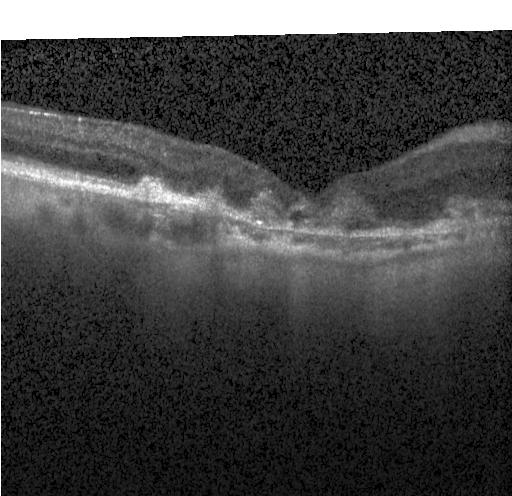 Retinal OCT cross-section showing choroidal neovascularization.